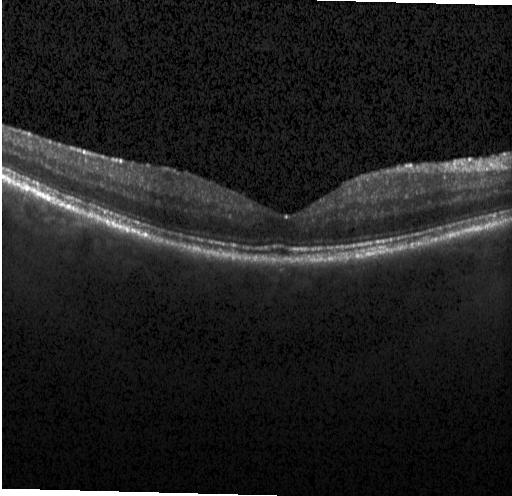

Heidelberg Spectralis OCT system. SD-OCT. Retinal OCT cross-section. Macular OCT: neither choroidal neovascularization, diabetic macular edema, nor drusen.